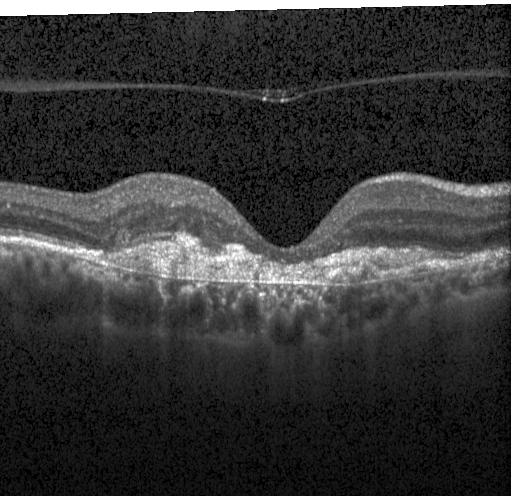

OCT scan showing CNV.